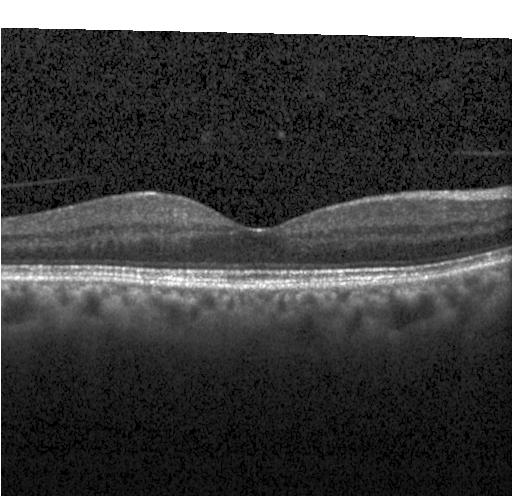
Spectral-domain optical coherence tomography, optical coherence tomography B-scan, Heidelberg Spectralis OCT system — Diagnosis: no evidence of choroidal neovascularization, diabetic macular edema, or drusen.